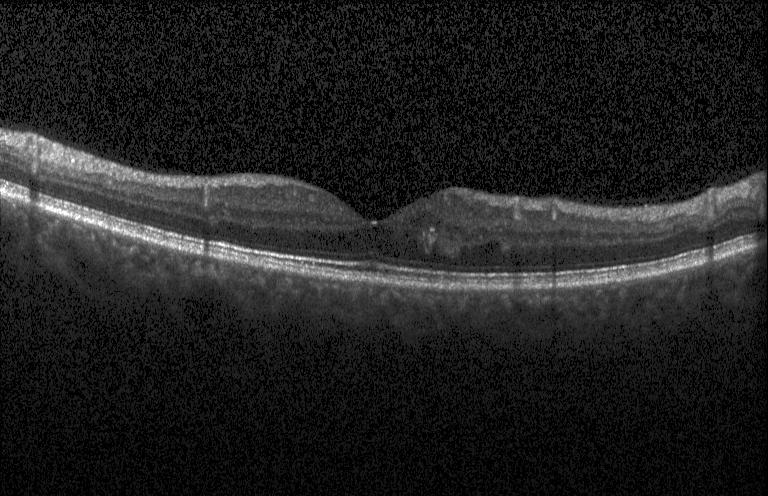
OCT finding: no evidence of choroidal neovascularization, diabetic macular edema, or drusen.